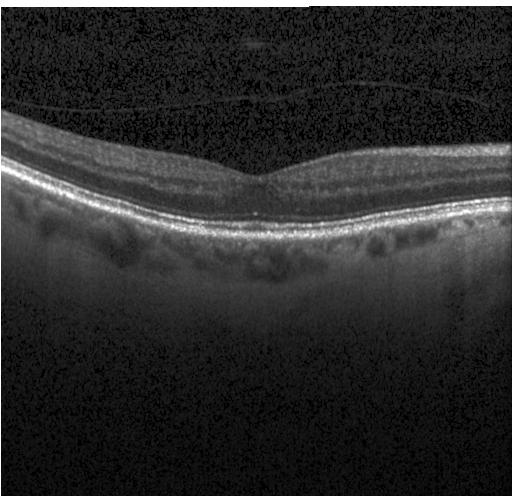

SD-OCT; acquired on a Heidelberg Spectralis; OCT B-scan.
Finding: no choroidal neovascularization, diabetic macular edema, or drusen.